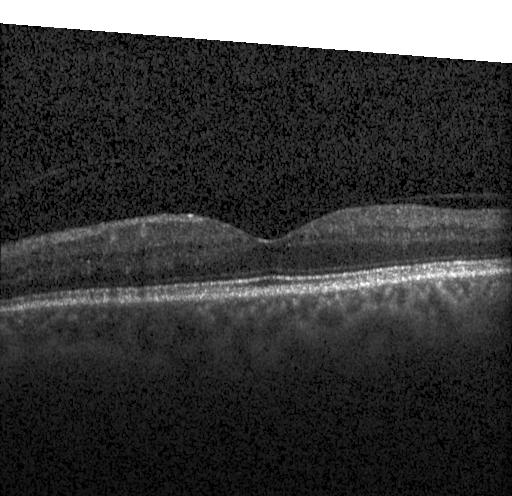
Retinal OCT cross-section; instrument: Heidelberg Spectralis; spectral-domain optical coherence tomography. Diagnosis: no CNV, no DME, and no drusen.